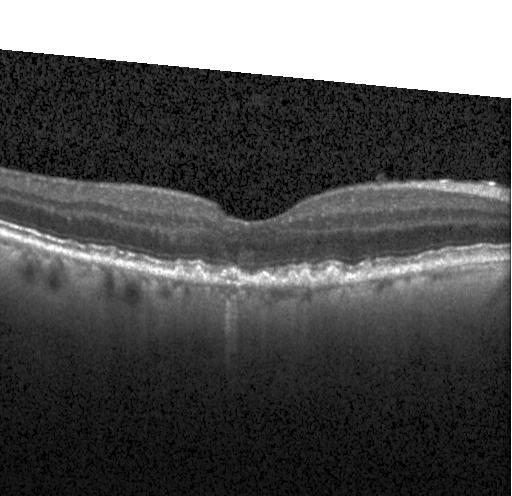

Fovea-centered. Heidelberg Spectralis OCT system. OCT line scan. Macular OCT: multiple drusen.